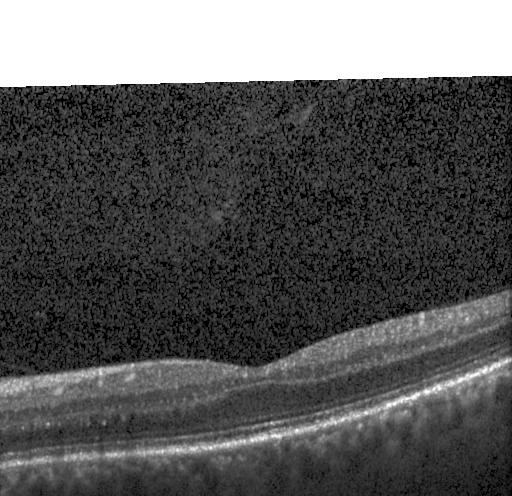 Impression: no choroidal neovascularization, no diabetic macular edema, and no drusen.